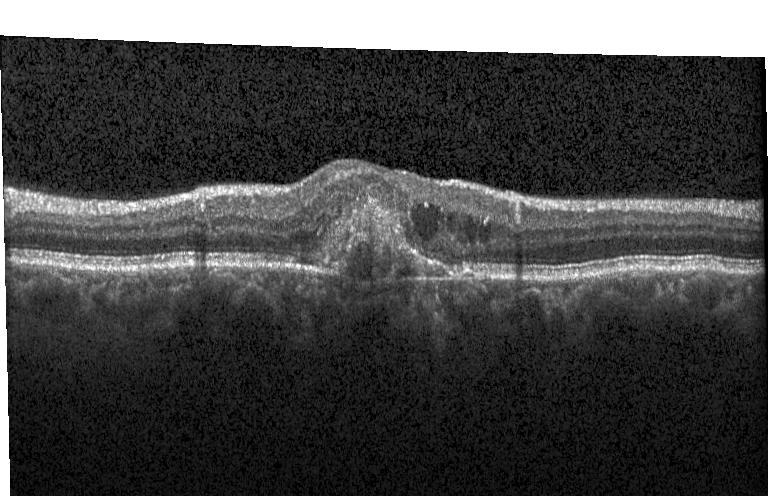
OCT finding: choroidal neovascularization (CNV).